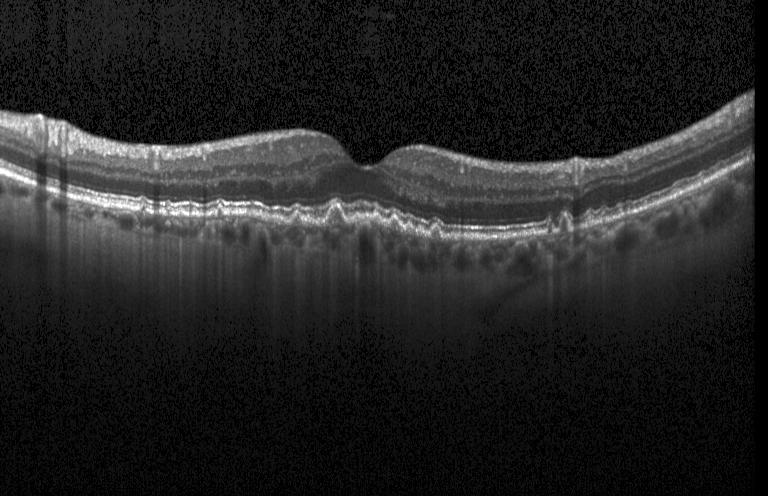
Retinal OCT B-scan. Diagnosis: multiple drusen.